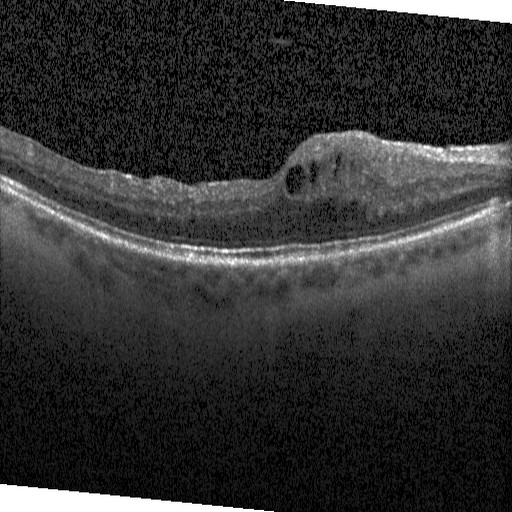

Optical coherence tomography B-scan, Heidelberg Spectralis OCT system
Impression: DME.